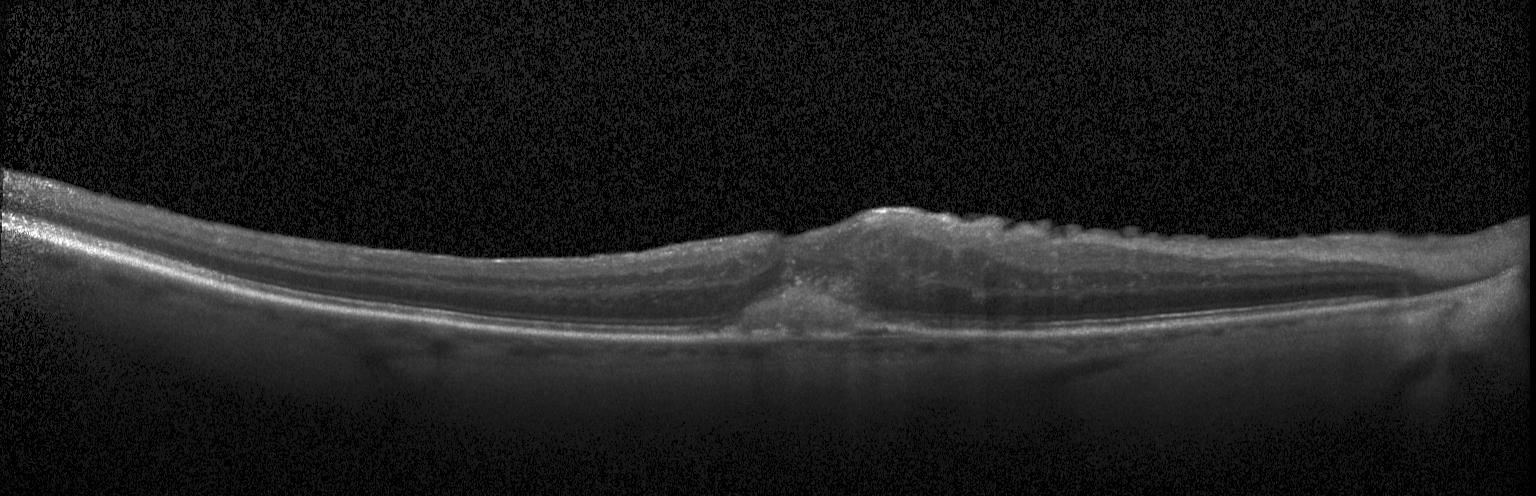
Instrument: Heidelberg Spectralis, OCT B-scan.
Diagnosis: choroidal neovascularization.